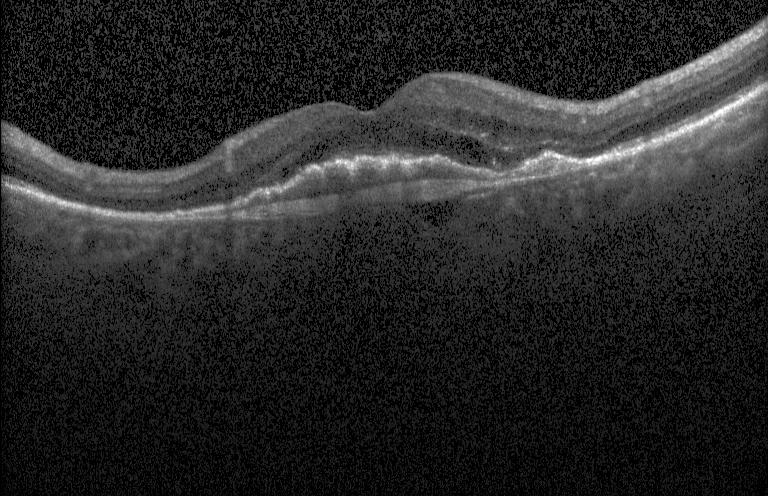

Assessment: a choroidal neovascular membrane.